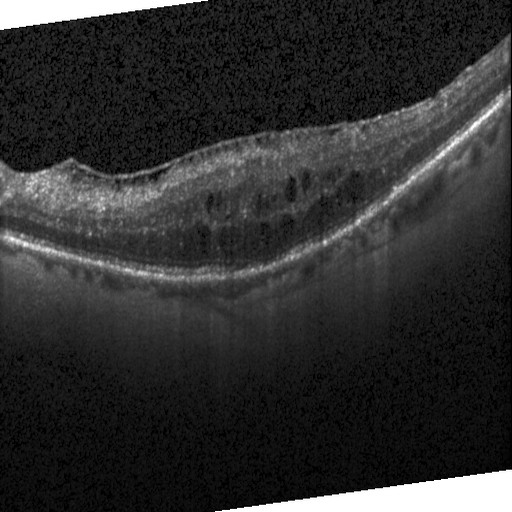 Centered on the fovea; OCT B-scan; Heidelberg Spectralis. Dx: diabetic macular edema (DME).